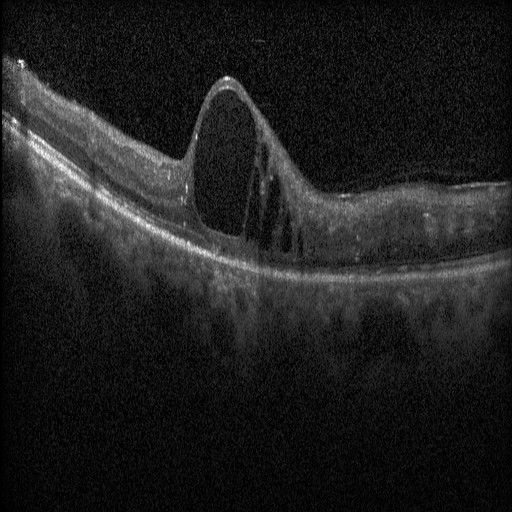

Macular OCT: diabetic macular edema (DME).